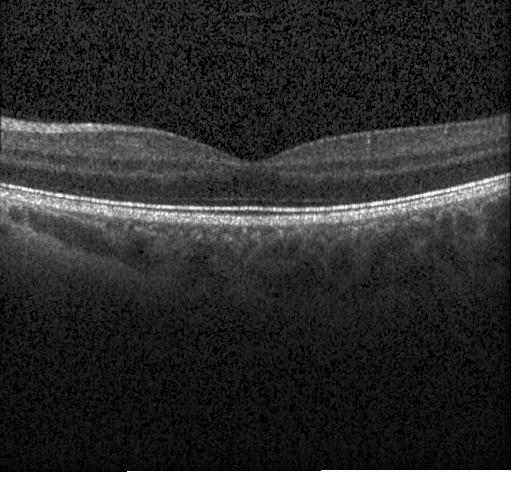

Instrument: Heidelberg Spectralis, optical coherence tomography scan.
Finding: no choroidal neovascularization, no diabetic macular edema, and no drusen.